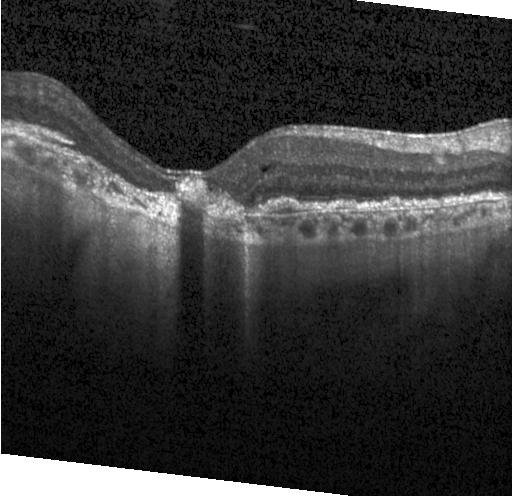

Centered on the fovea. Spectral-domain OCT. Heidelberg Spectralis OCT system. Retinal OCT cross-section.
Finding: a choroidal neovascular membrane.